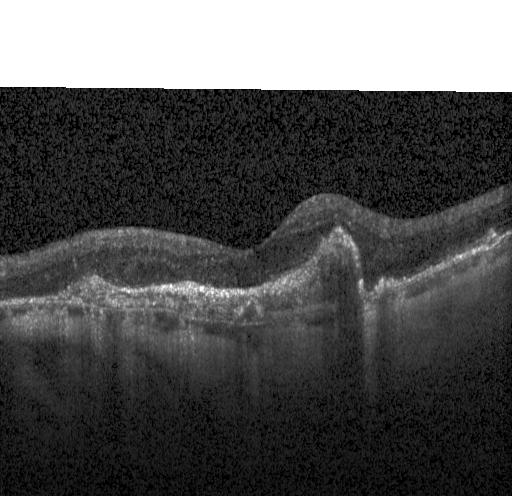 Centered on the fovea · spectral-domain OCT · optical coherence tomography scan — Impression: choroidal neovascularization.